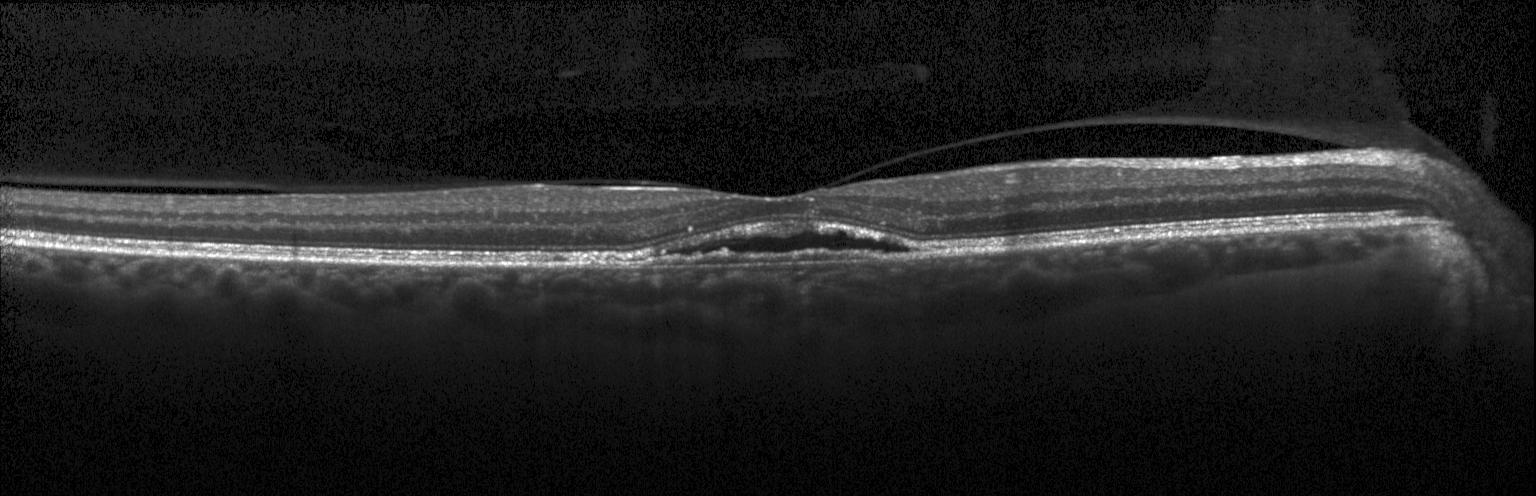
This B-scan demonstrates choroidal neovascularization (CNV).